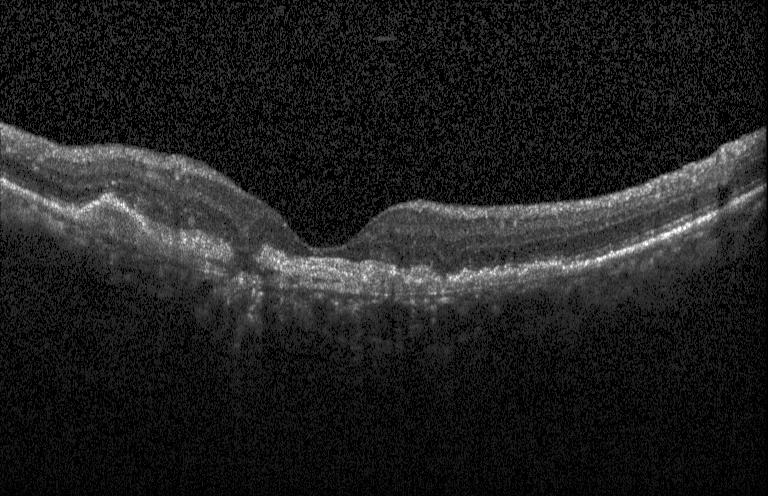
Acquired on a Heidelberg Spectralis, horizontal scan through the fovea, retinal OCT B-scan, SD-OCT. Finding: a choroidal neovascular membrane.